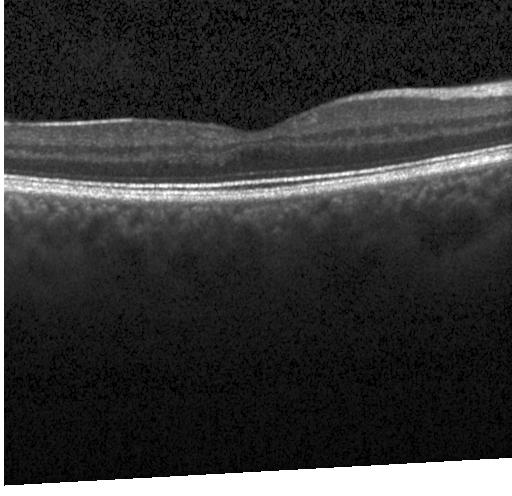
Instrument: Heidelberg Spectralis; spectral-domain OCT; centered on the fovea; retinal OCT cross-section.
Diagnosis: no CNV, no DME, and no drusen.